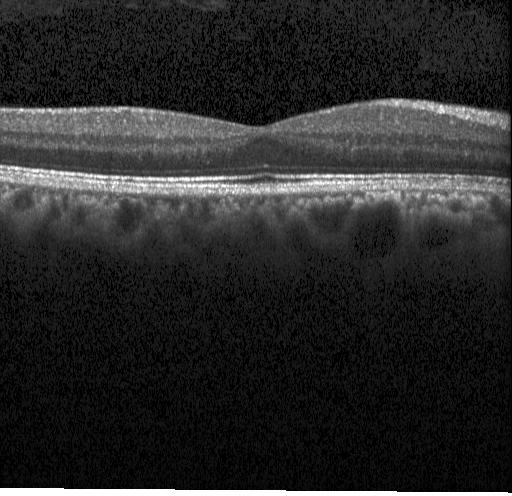 Macular OCT demonstrating no CNV, DME, or drusen.